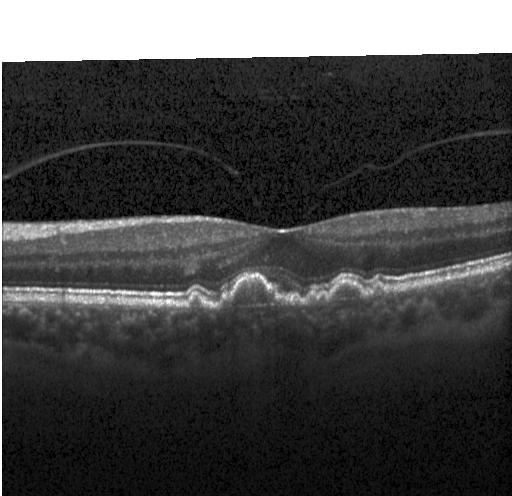

Retinal OCT cross-section
OCT finding: sub-RPE drusenoid deposits.